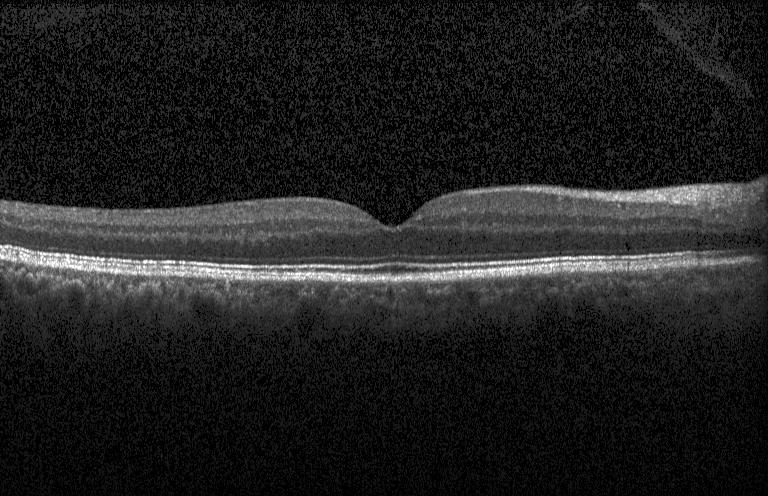
Retinal OCT B-scan.
Assessment: neither choroidal neovascularization, diabetic macular edema, nor drusen.